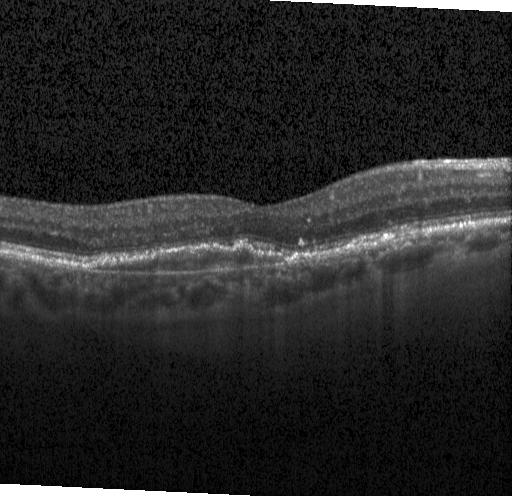 Macular scan; OCT B-scan; spectral-domain optical coherence tomography; instrument: Heidelberg Spectralis
Finding: choroidal neovascularization (CNV).